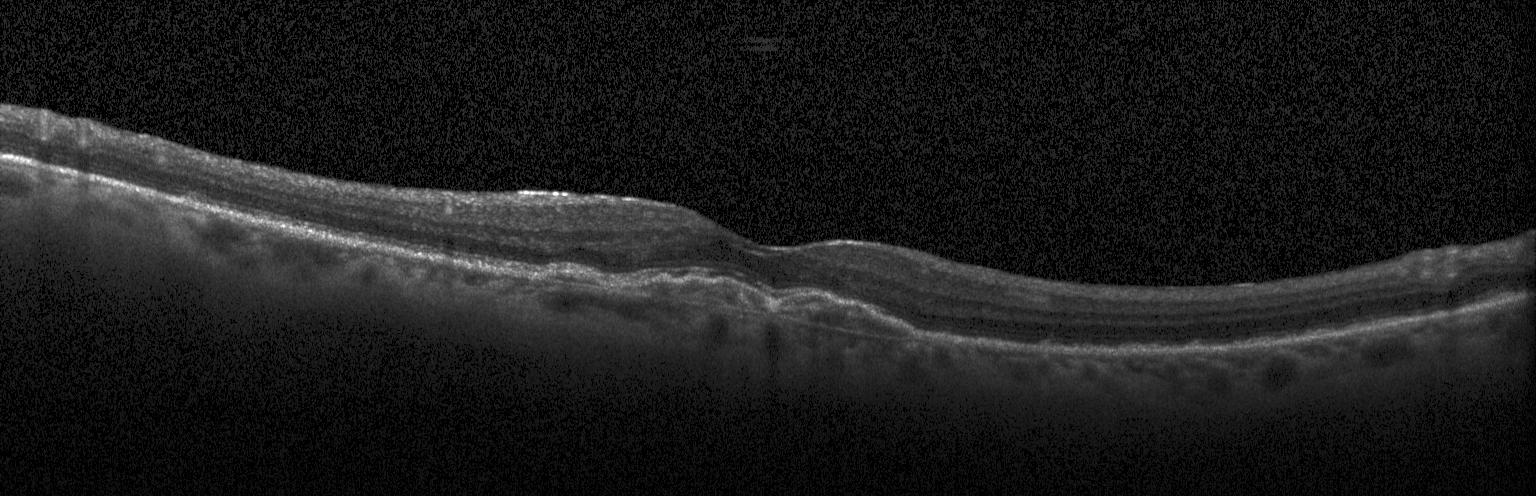
Retinal OCT cross-section. Finding: choroidal neovascularization.